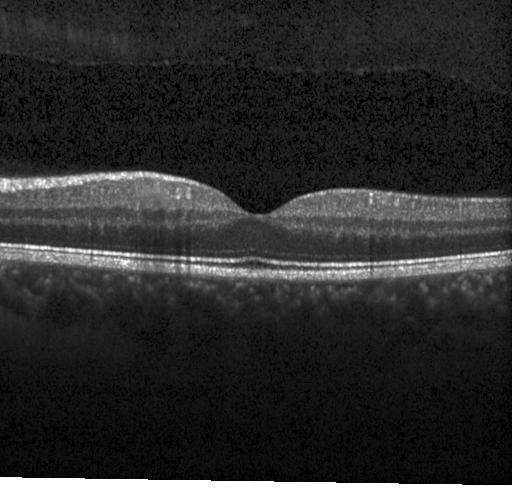

Dx: no choroidal neovascularization, diabetic macular edema, or drusen.